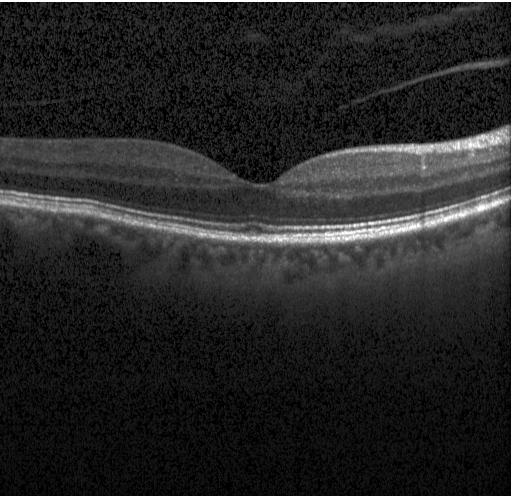
Diagnosis: no choroidal neovascularization, no diabetic macular edema, and no drusen.